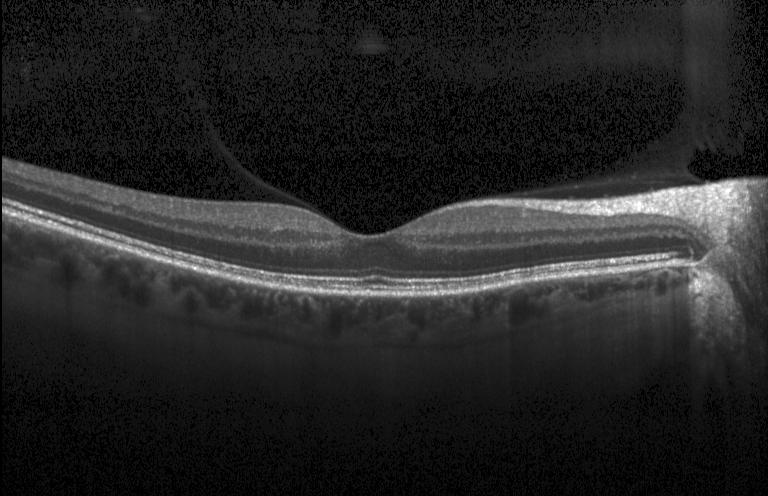
No CNV, no DME, and no drusen.